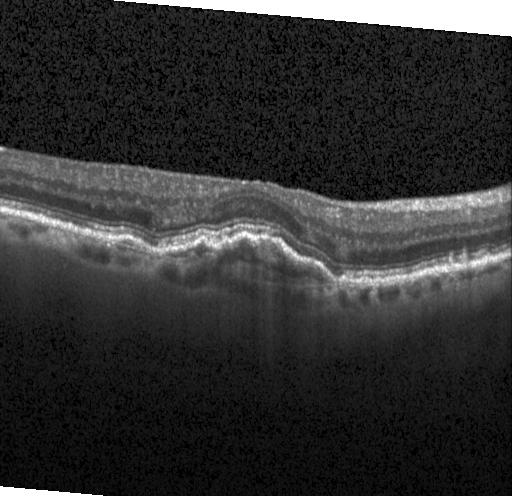

Heidelberg Spectralis; retinal OCT cross-section; SD-OCT. Assessment: a choroidal neovascular membrane.